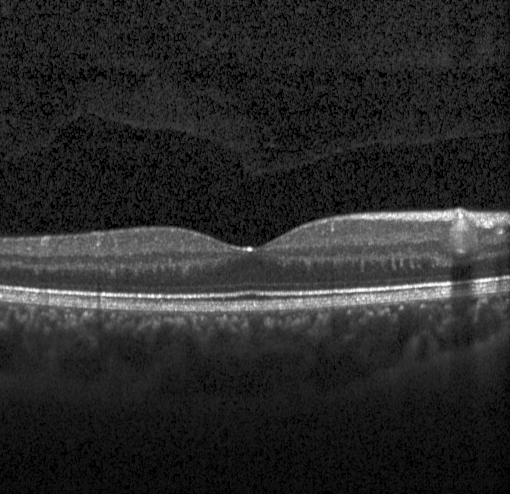
Retinal OCT cross-section
Dx: neither choroidal neovascularization, diabetic macular edema, nor drusen.